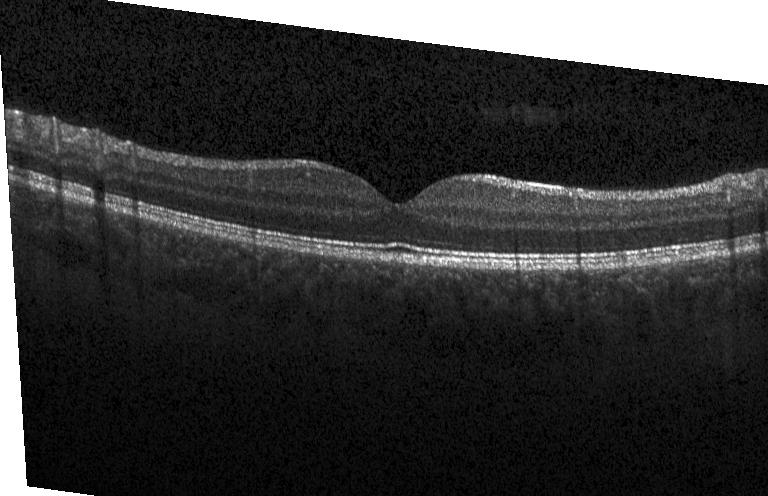

SD-OCT. Horizontal scan through the fovea. Retinal OCT B-scan. Heidelberg Spectralis.
Diagnosis: neither choroidal neovascularization, diabetic macular edema, nor drusen.